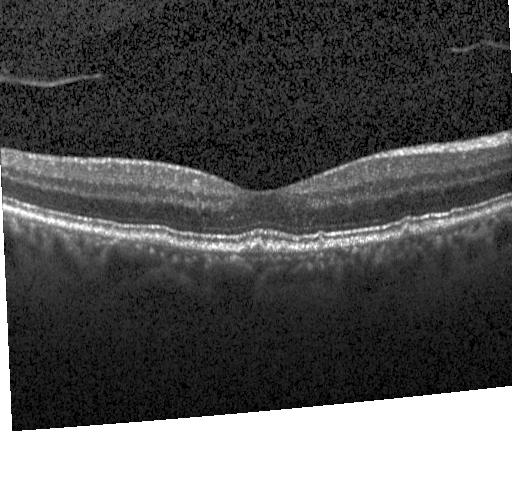
Heidelberg Spectralis OCT system · retinal OCT cross-section.
Drusen.